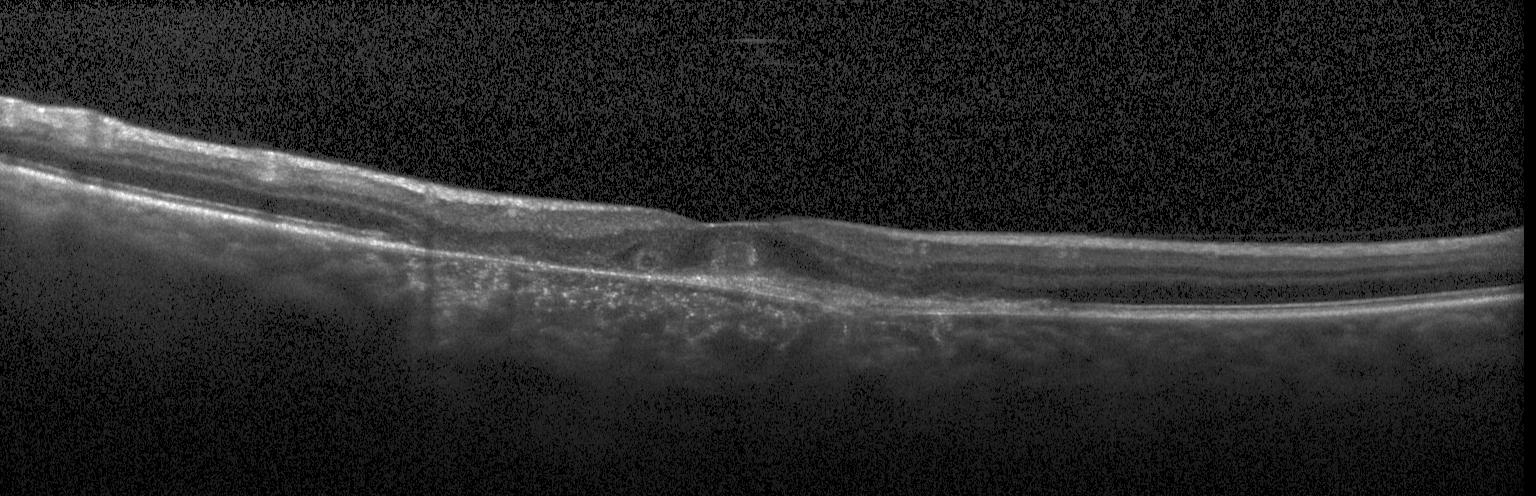 Spectral-domain OCT · horizontal scan through the fovea · optical coherence tomography B-scan. A choroidal neovascular membrane.